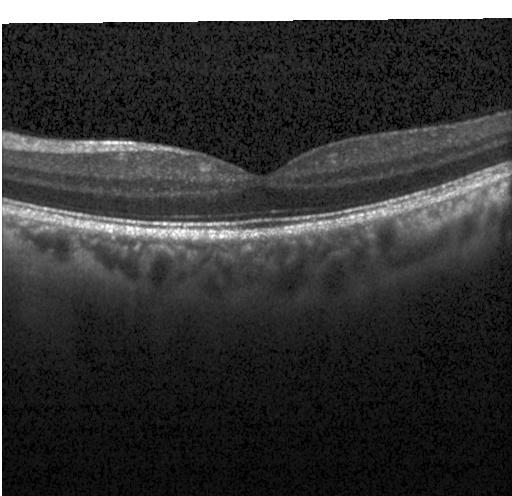
Spectral-domain OCT. Retinal OCT cross-section. Heidelberg Spectralis. Macular scan
Impression: no choroidal neovascularization, diabetic macular edema, or drusen.